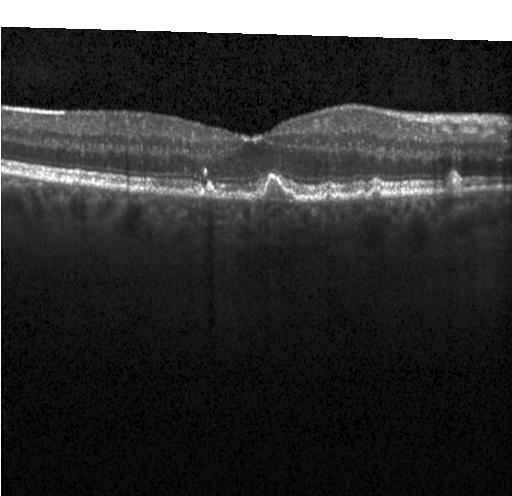 Acquired on a Heidelberg Spectralis · centered on the fovea · retinal OCT B-scan · spectral-domain optical coherence tomography
Macular OCT: sub-RPE drusenoid deposits.